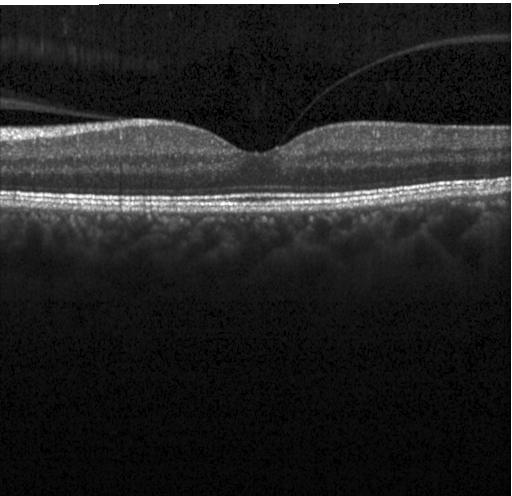 OCT B-scan, spectral-domain OCT, instrument: Heidelberg Spectralis, centered on the fovea.
The scan shows no choroidal neovascularization, no diabetic macular edema, and no drusen.